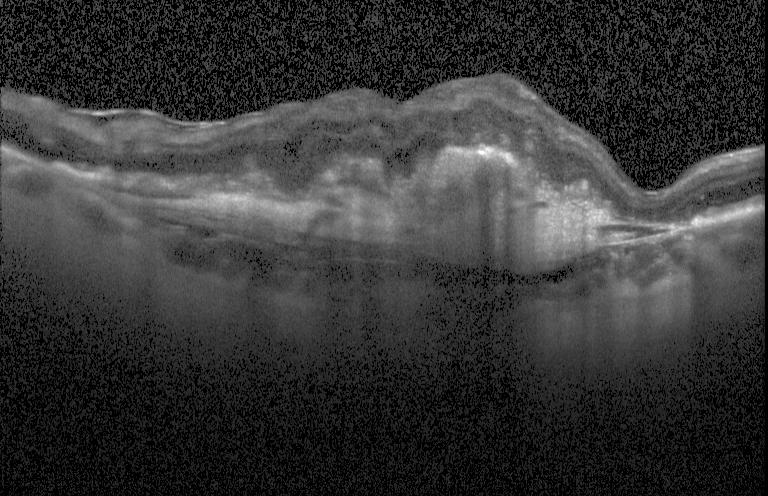 OCT line scan.
Diagnosis: choroidal neovascularization (CNV).